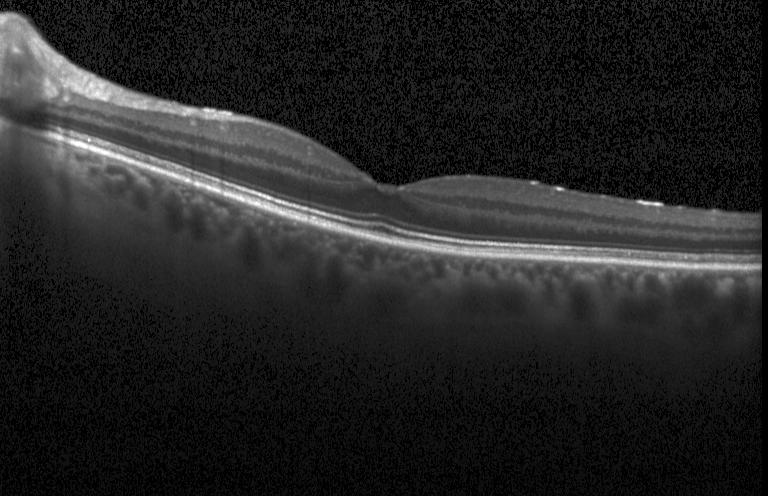 Finding: no choroidal neovascularization, diabetic macular edema, or drusen.